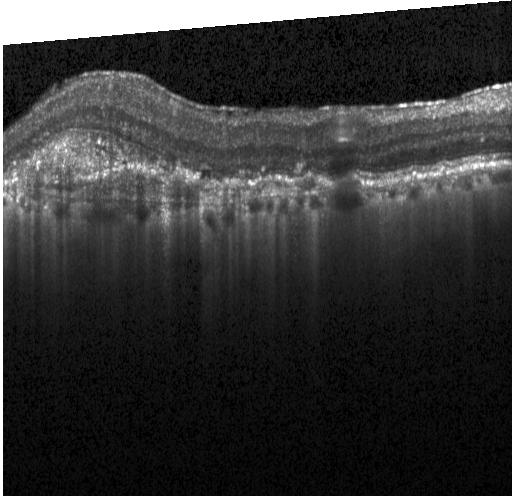 Dx: choroidal neovascularization (CNV).